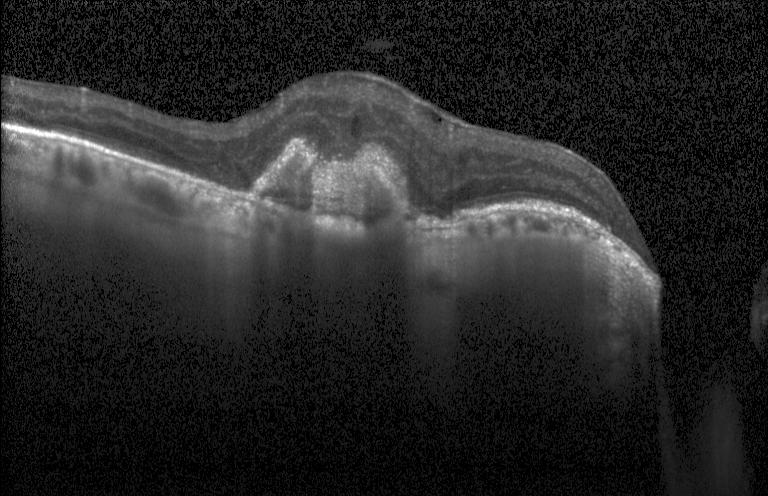
Optical coherence tomography scan, fovea-centered.
Diagnosis: a choroidal neovascular membrane.